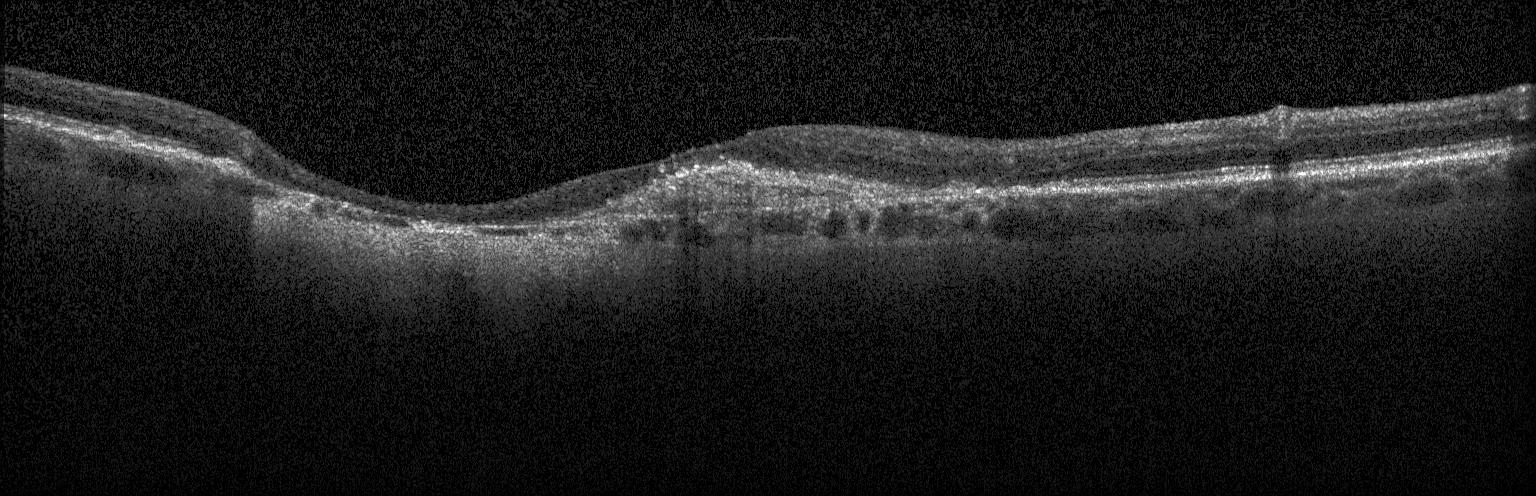 Diagnosis: choroidal neovascularization.